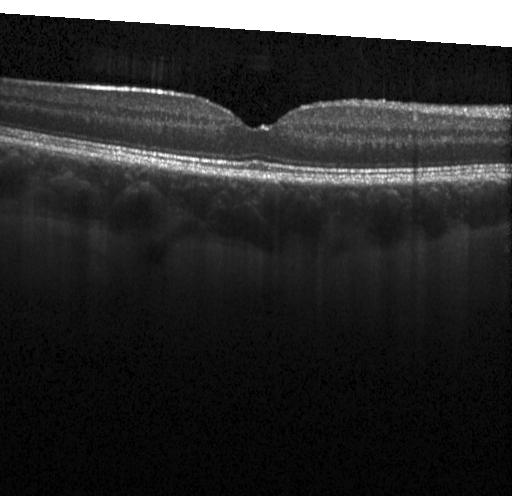
Retinal OCT cross-section — Dx: no choroidal neovascularization, no diabetic macular edema, and no drusen.